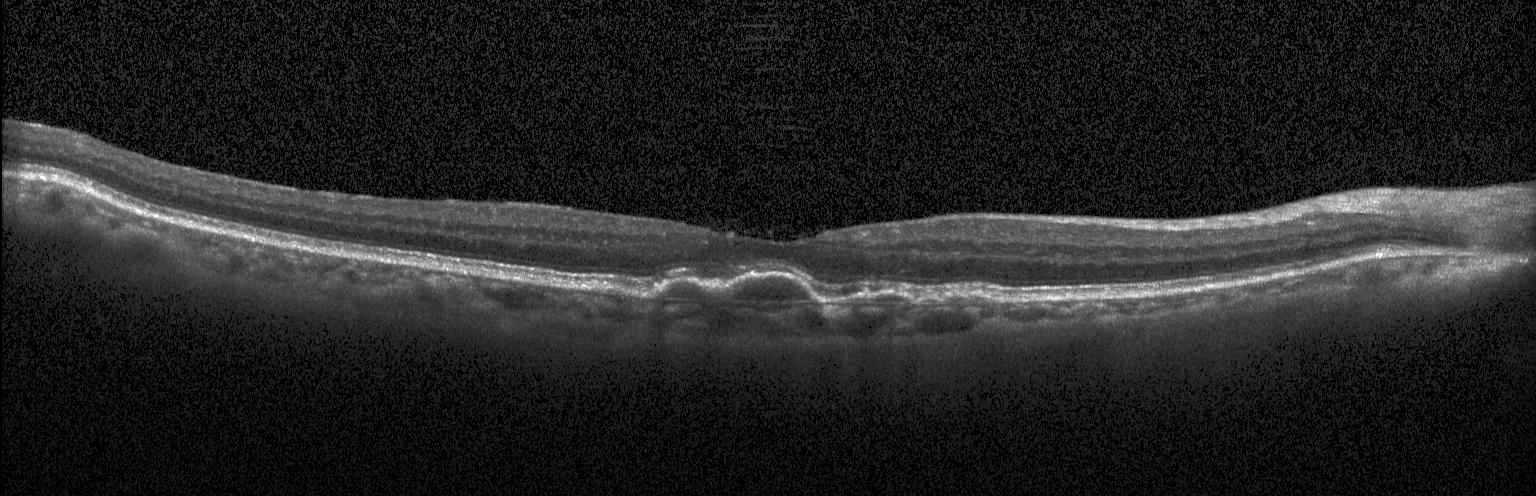 Centered on the fovea · spectral-domain optical coherence tomography · Heidelberg Spectralis · optical coherence tomography B-scan. Impression: a choroidal neovascular membrane.